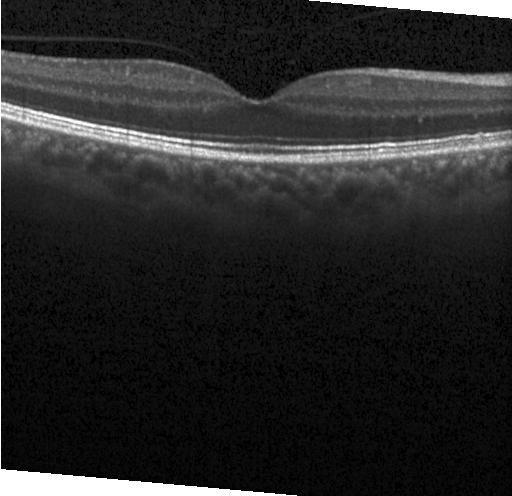

SD-OCT; acquired on a Heidelberg Spectralis; retinal OCT B-scan
The scan shows no choroidal neovascularization, diabetic macular edema, or drusen.